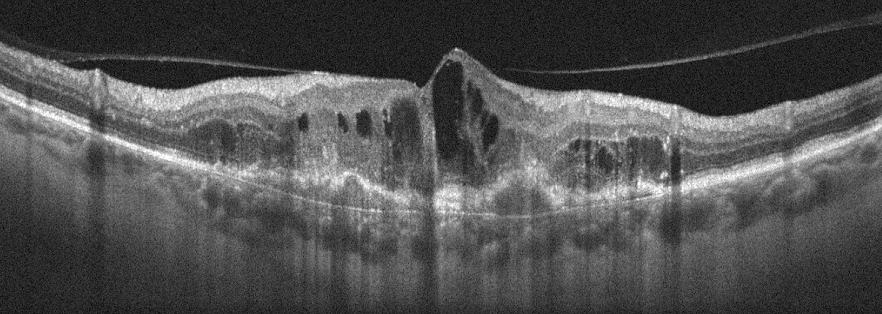 Optical coherence tomography B-scan. Impression: age-related macular degeneration.